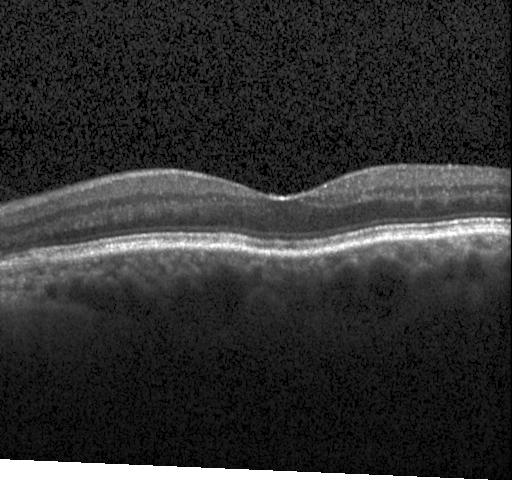
Impression: neither choroidal neovascularization, diabetic macular edema, nor drusen.